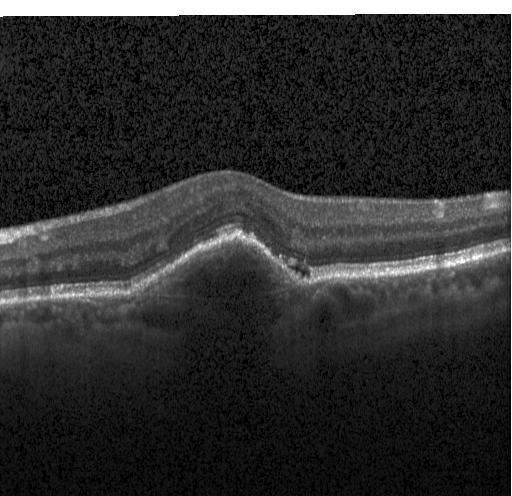 Retinal OCT B-scan
Macular OCT: choroidal neovascularization (CNV).